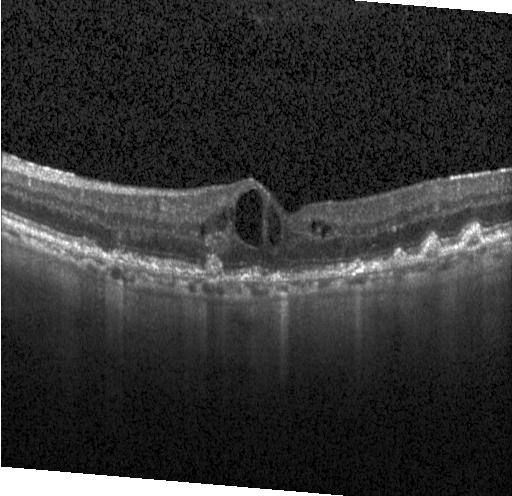

Retinal OCT cross-section · through the macula — Finding: choroidal neovascularization (CNV).